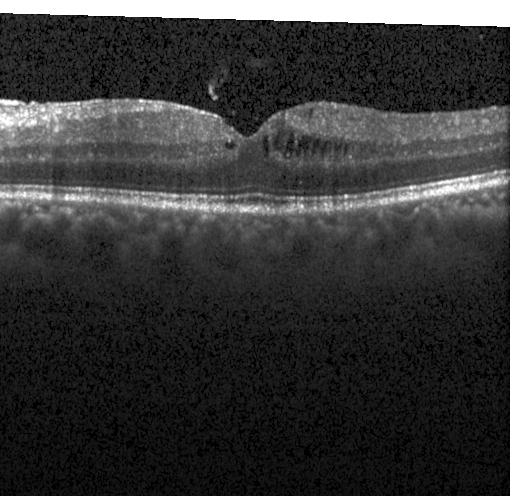

Retinal OCT cross-section showing DME.